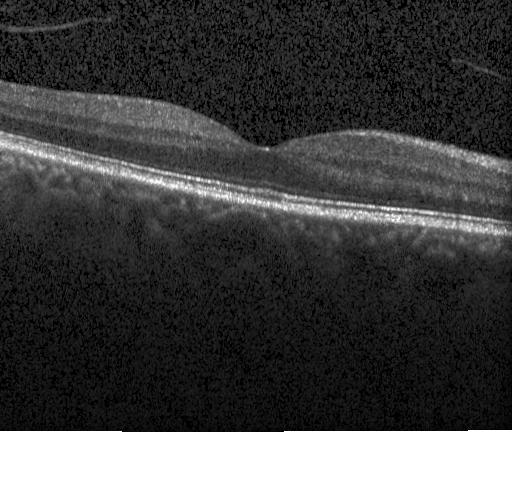 Retinal OCT cross-section. Heidelberg Spectralis OCT system. Fovea-centered.
Assessment: no CNV, DME, or drusen.